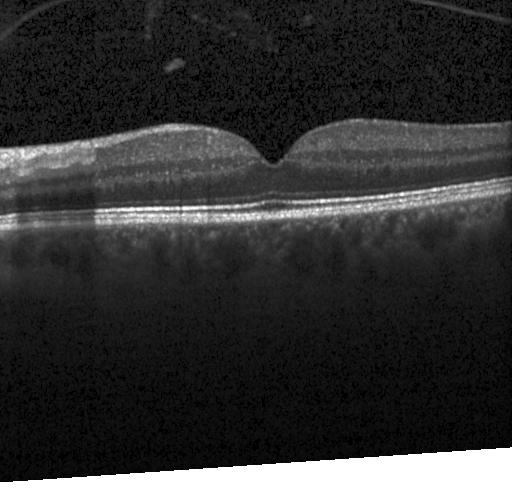

Retinal OCT B-scan, fovea-centered, spectral-domain optical coherence tomography, Heidelberg Spectralis OCT system.
Dx: no choroidal neovascularization, diabetic macular edema, or drusen.